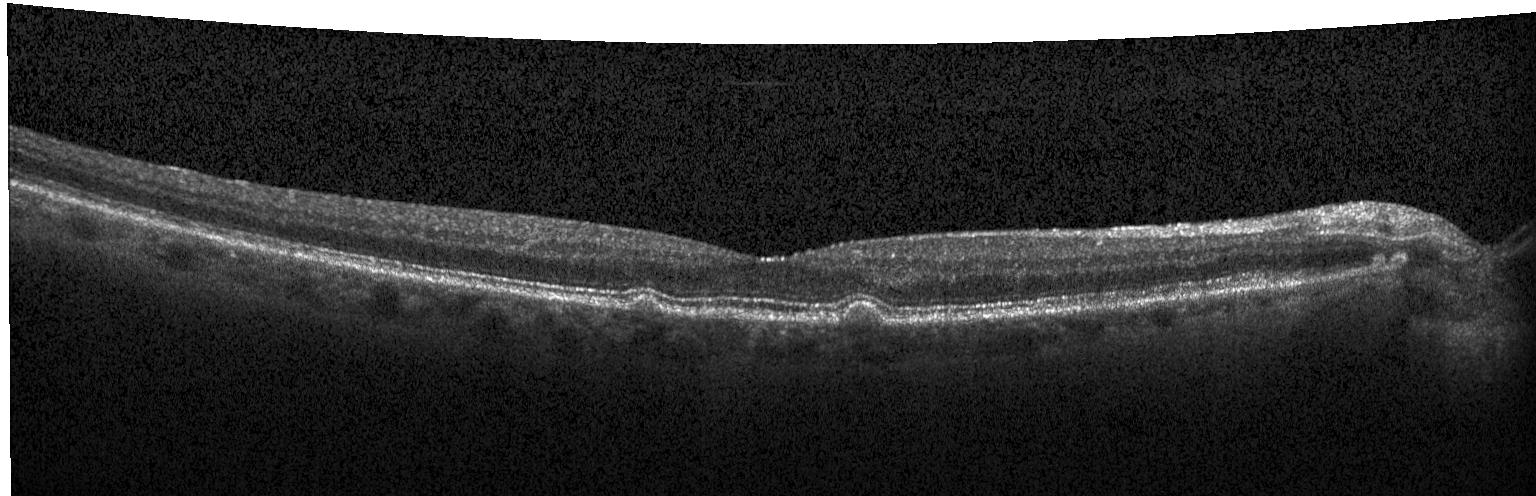

Through the macula · retinal OCT B-scan · Heidelberg Spectralis OCT system · SD-OCT. Finding: multiple drusen.